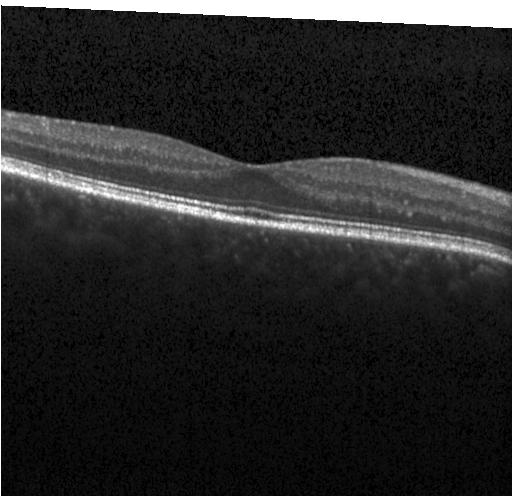

Macular OCT: no choroidal neovascularization, diabetic macular edema, or drusen.